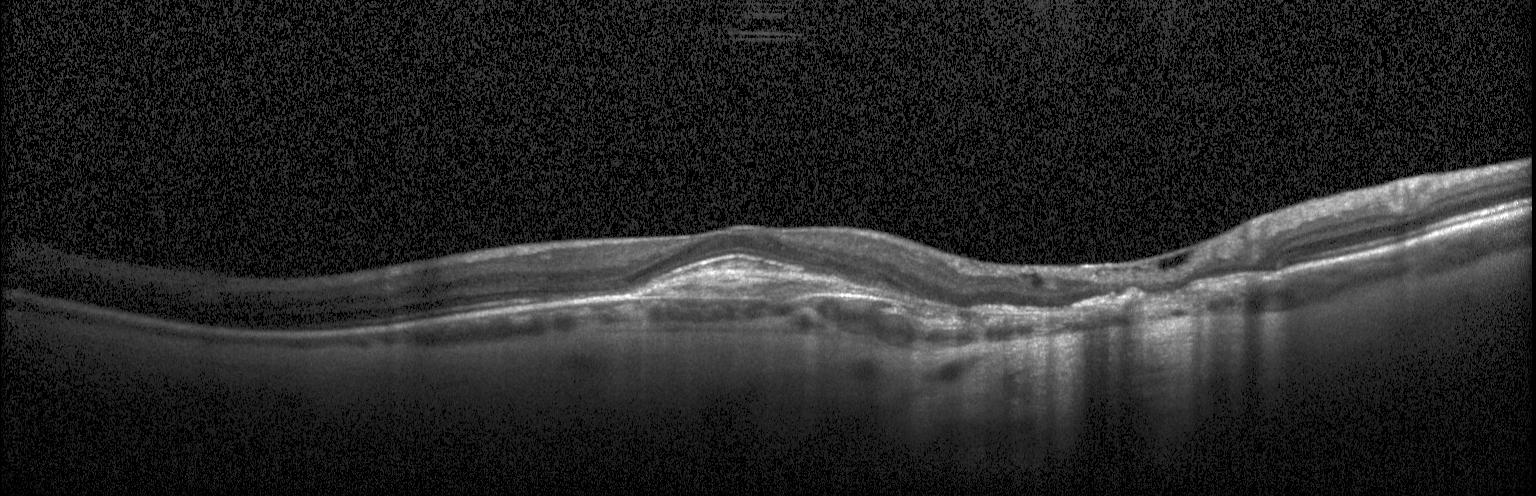
Optical coherence tomography B-scan. Finding: choroidal neovascularization (CNV).